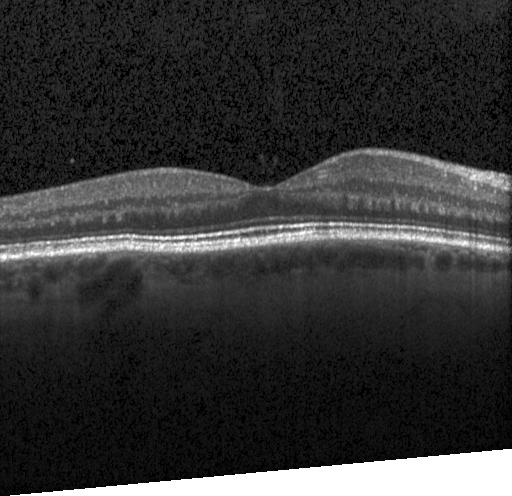
OCT scan showing neither CNV, DME, nor drusen.